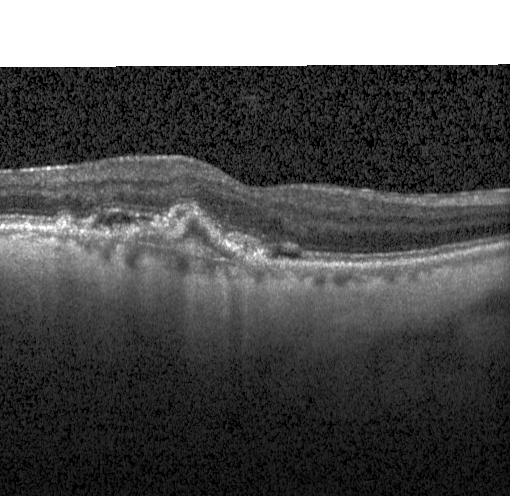
Dx: a choroidal neovascular membrane.